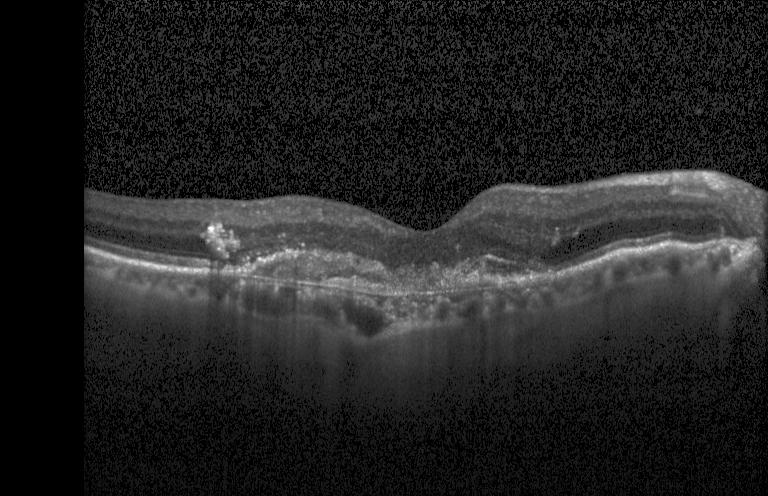

Finding: choroidal neovascularization.